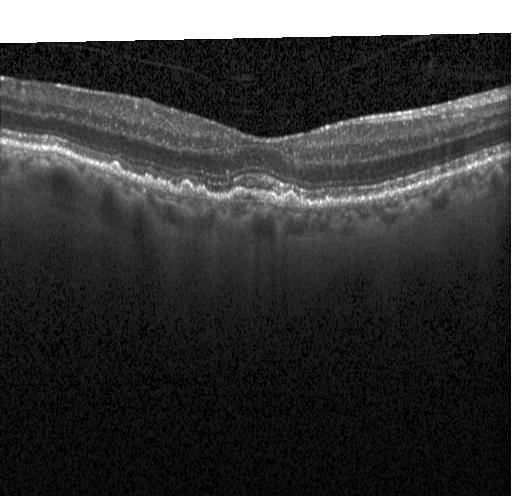 SD-OCT · optical coherence tomography scan · macular scan. Diagnosis: a choroidal neovascular membrane.